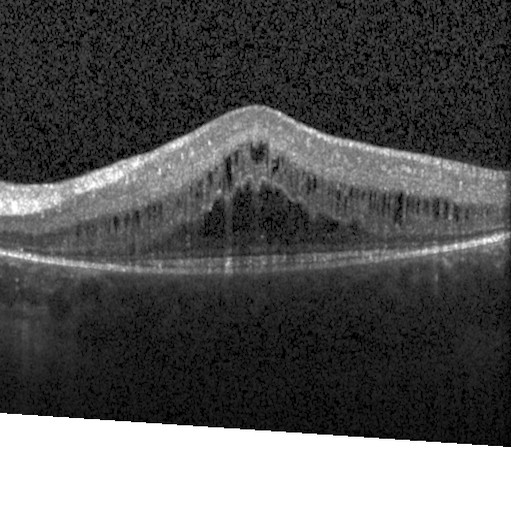 OCT B-scan; SD-OCT. Impression: diabetic macular edema.